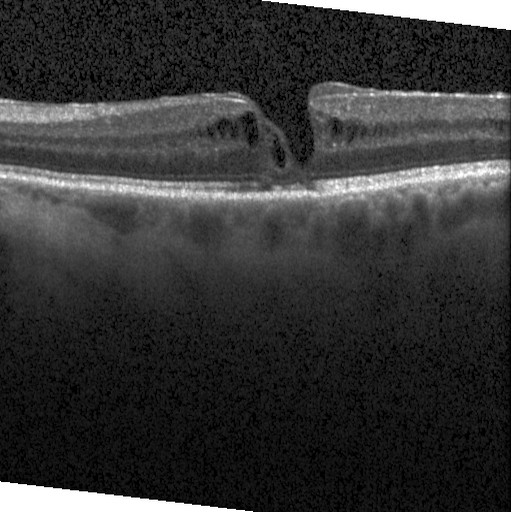

OCT line scan. Diagnosis: diabetic macular edema.